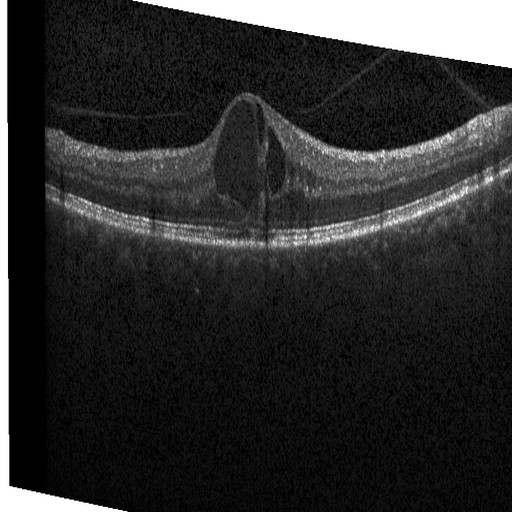 Optical coherence tomography scan. Spectral-domain OCT. Heidelberg Spectralis OCT system
Diabetic macular edema.